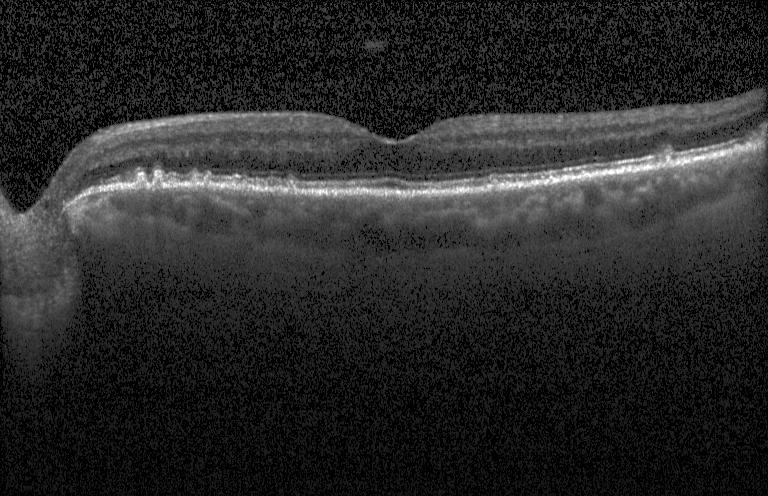

Retinal OCT B-scan
Macular OCT: drusen.